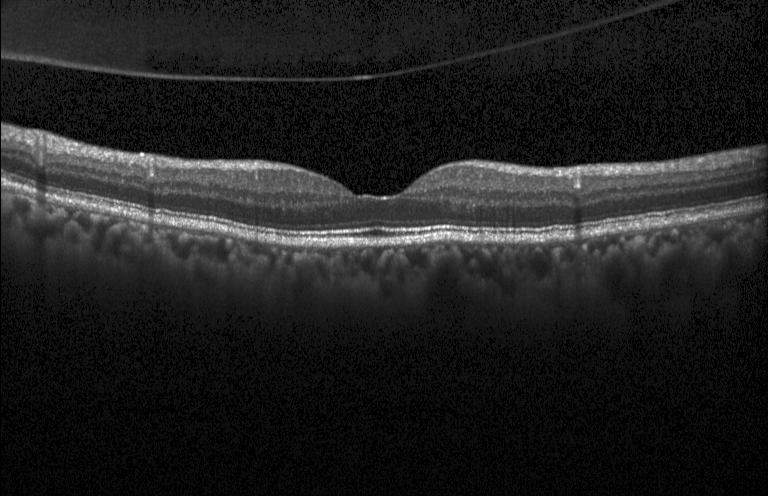 Finding: no evidence of CNV, DME, or drusen.